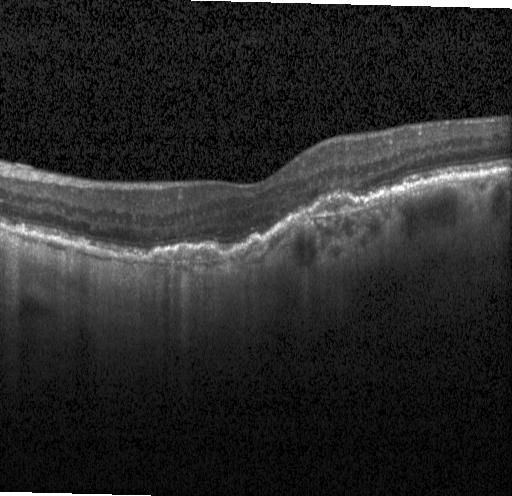

OCT line scan; Heidelberg Spectralis OCT system; spectral-domain OCT. Finding: CNV.